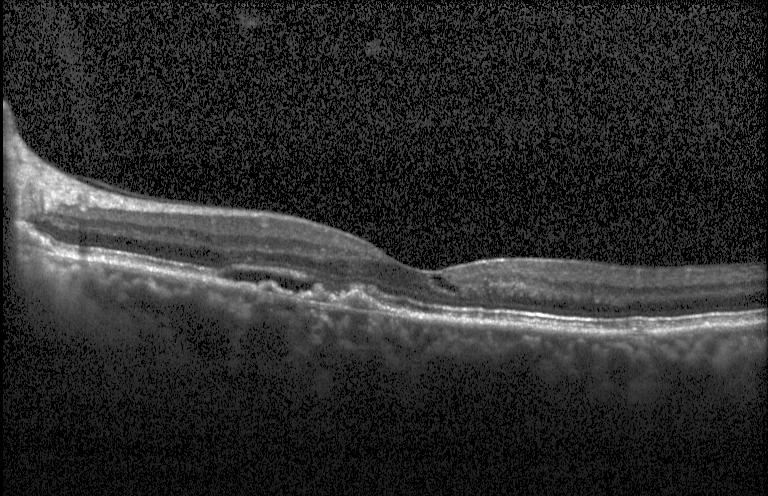
Through the macula, optical coherence tomography B-scan
Assessment: a choroidal neovascular membrane.